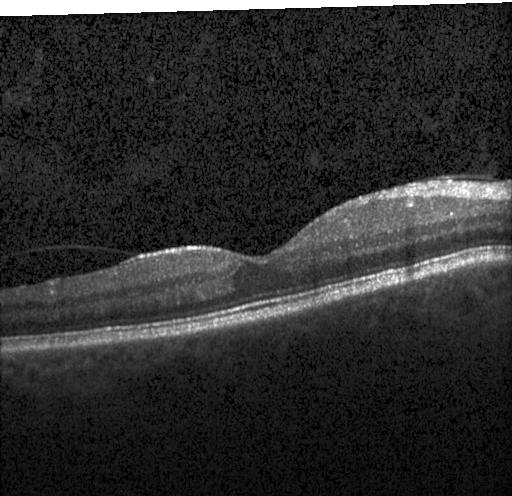

Retinal OCT cross-section · Heidelberg Spectralis · fovea-centered · SD-OCT — Assessment: no choroidal neovascularization, no diabetic macular edema, and no drusen.